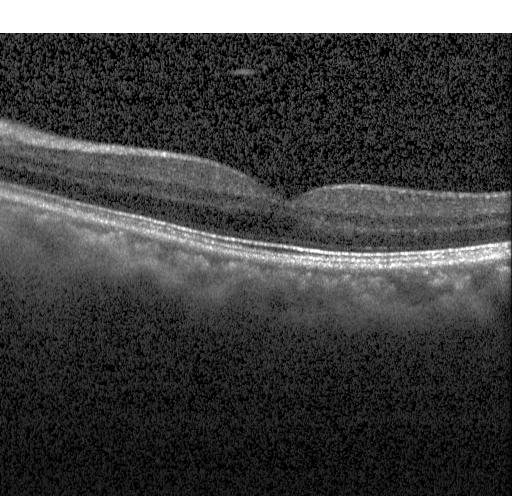 Finding: no evidence of choroidal neovascularization, diabetic macular edema, or drusen.